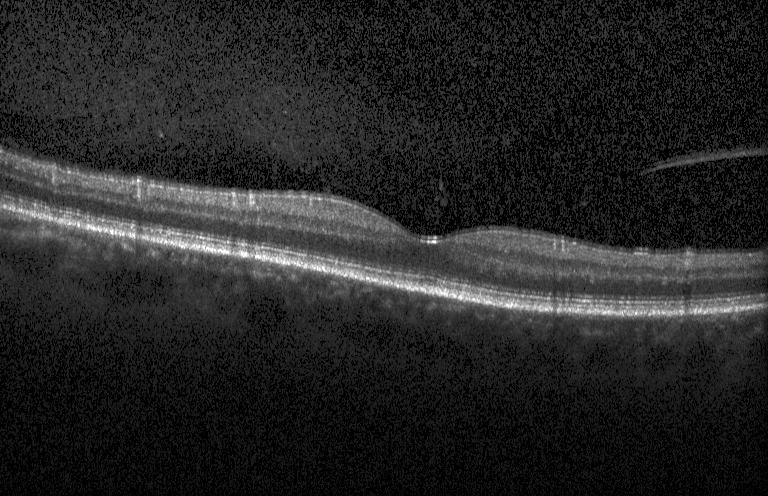
Dx: neither CNV, DME, nor drusen.